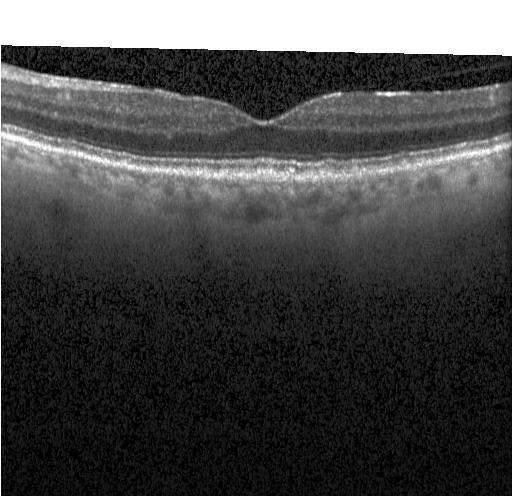
Retinal OCT B-scan.
Macular OCT: drusen.